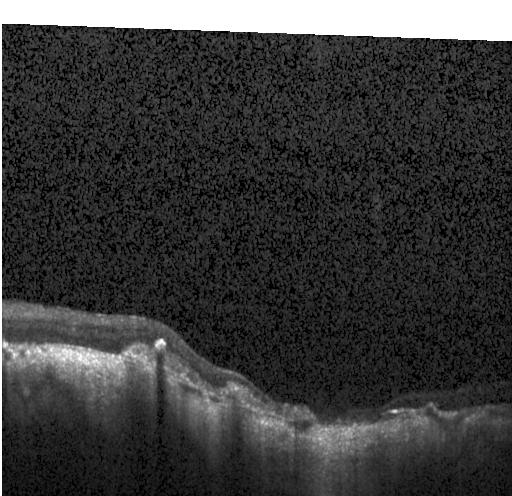 Impression: a choroidal neovascular membrane.